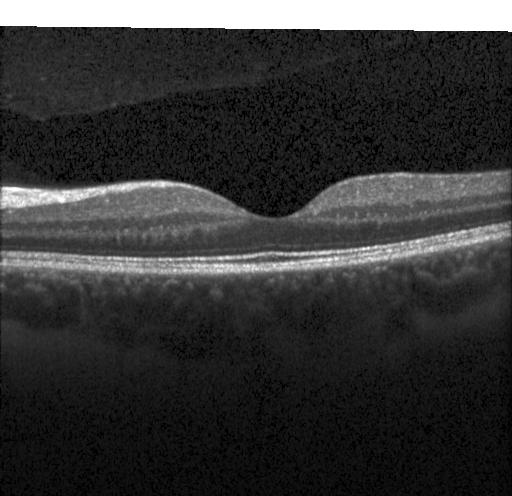

OCT B-scan; through the macula; spectral-domain optical coherence tomography; instrument: Heidelberg Spectralis.
Diagnosis: no evidence of CNV, DME, or drusen.